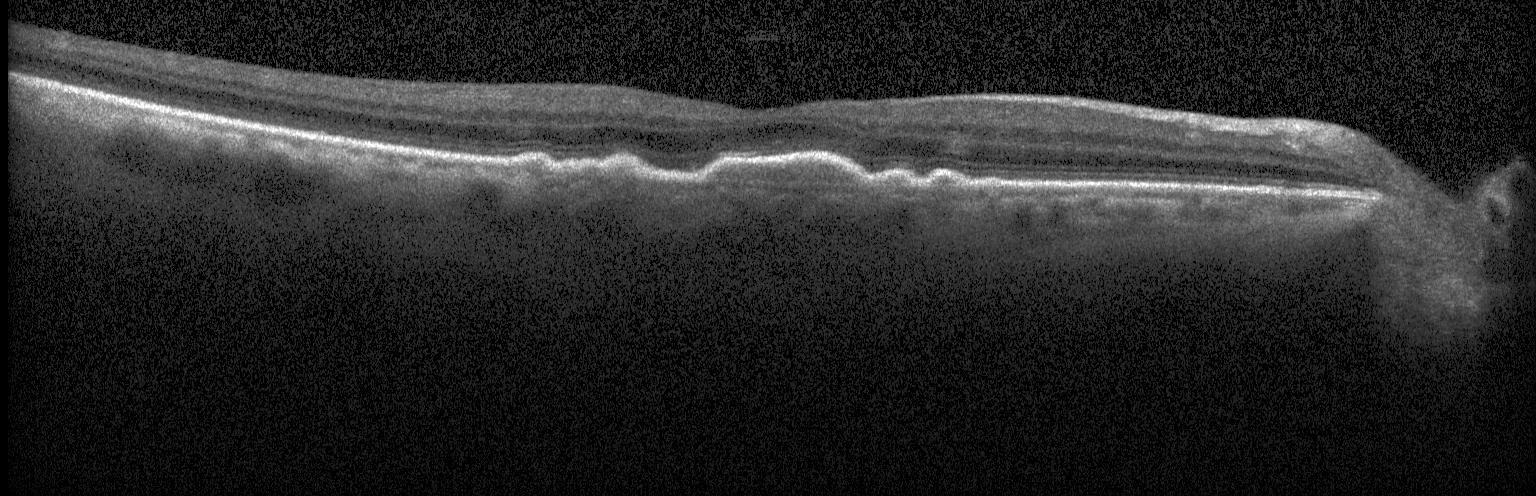
Macular OCT: CNV.